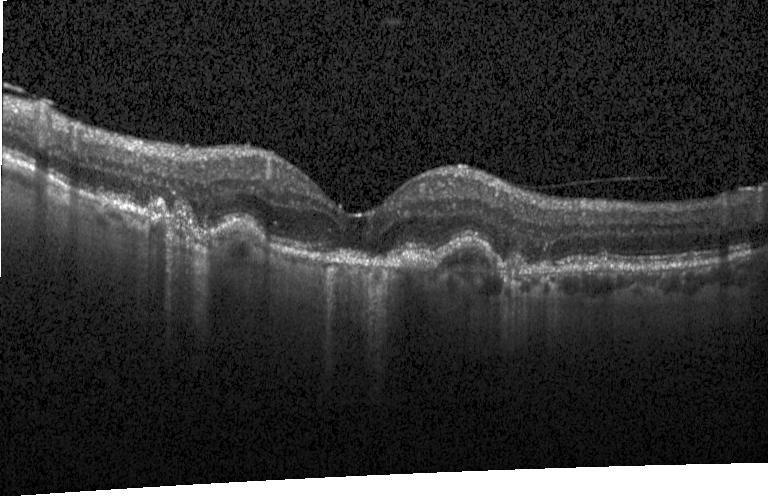 Retinal OCT B-scan — This B-scan demonstrates CNV.